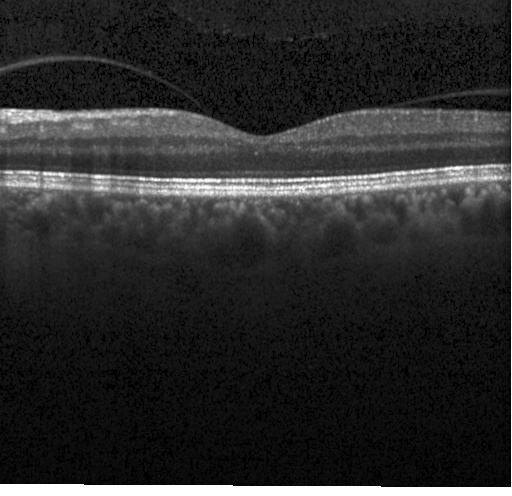

Finding: no evidence of CNV, DME, or drusen.